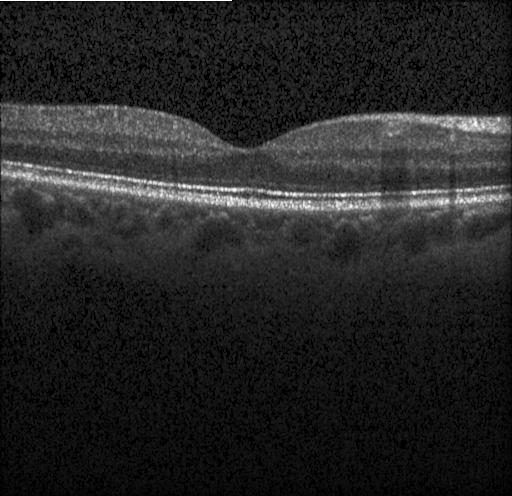
Retinal OCT cross-section — Macular OCT: no choroidal neovascularization, diabetic macular edema, or drusen.